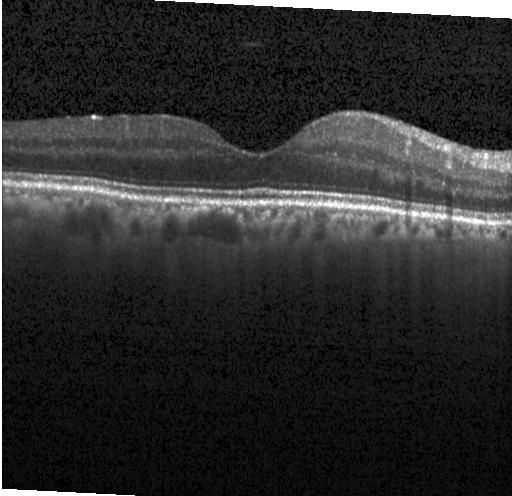

Spectral-domain optical coherence tomography; retinal OCT cross-section — OCT finding: no evidence of choroidal neovascularization, diabetic macular edema, or drusen.